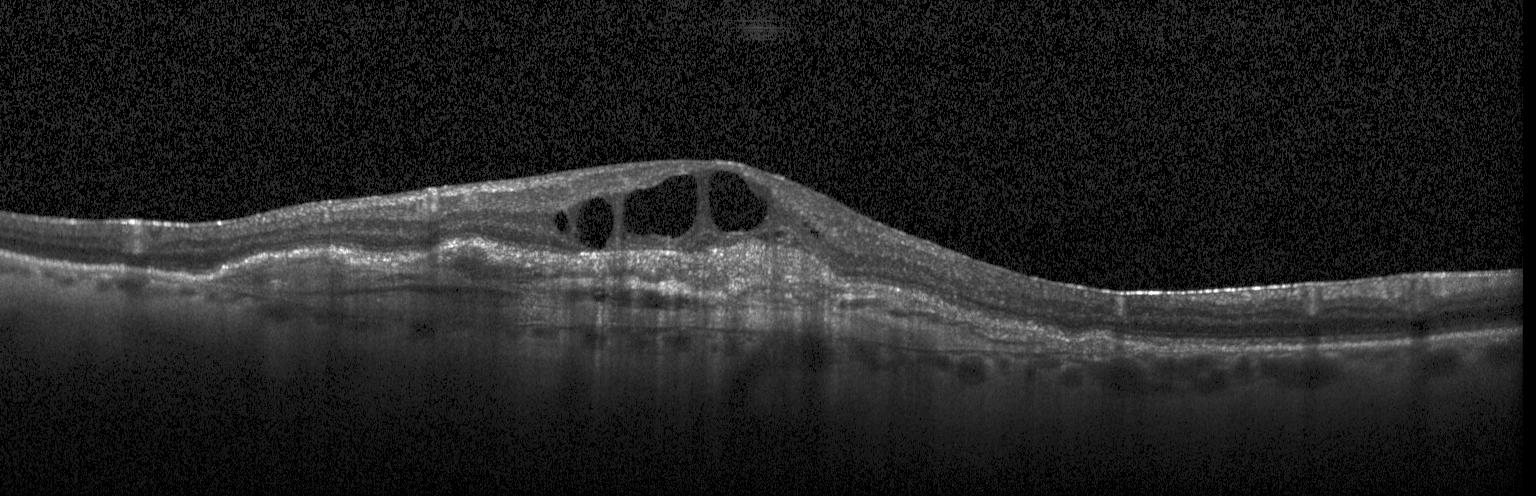

Optical coherence tomography scan. Through the macula. Spectral-domain optical coherence tomography — Macular OCT: choroidal neovascularization (CNV).